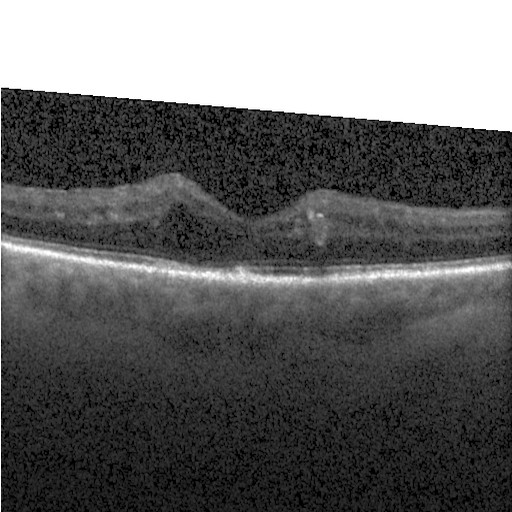

Impression: diabetic macular edema.